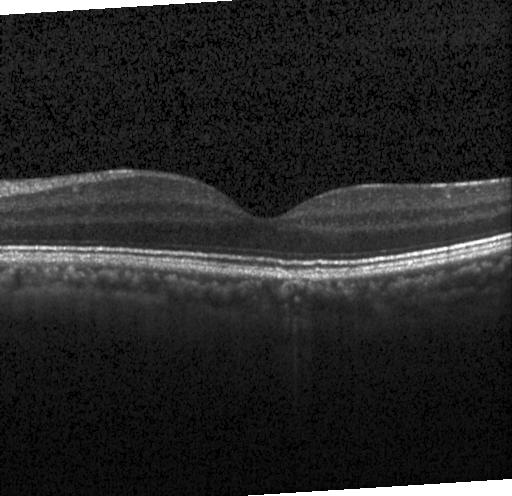

Finding: neither choroidal neovascularization, diabetic macular edema, nor drusen.